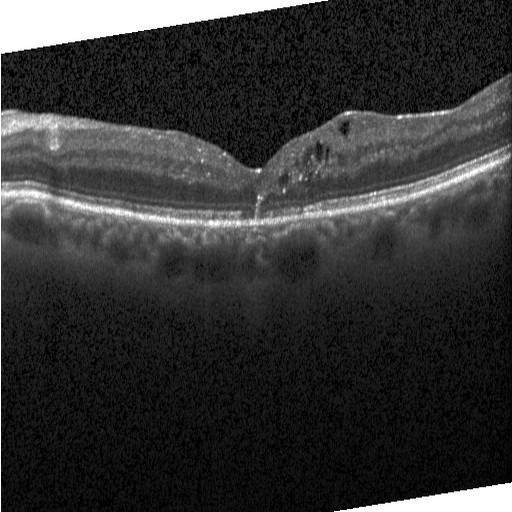 OCT finding: diabetic macular edema.